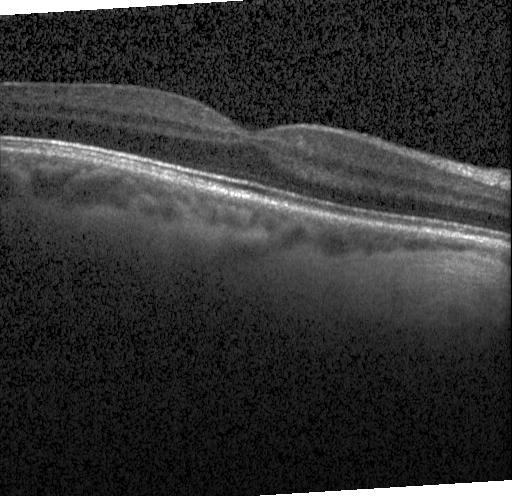

OCT line scan, SD-OCT, Heidelberg Spectralis
Impression: no evidence of choroidal neovascularization, diabetic macular edema, or drusen.